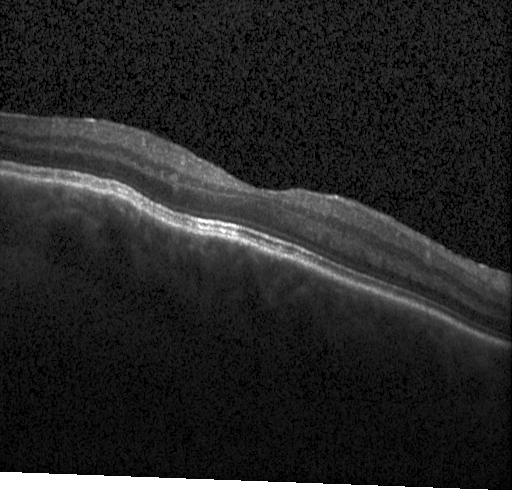
Assessment: no CNV, no DME, and no drusen.